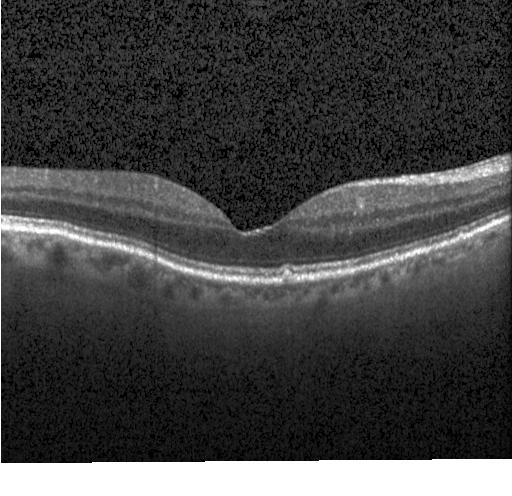
Fovea-centered, OCT line scan, spectral-domain optical coherence tomography. The scan shows neither CNV, DME, nor drusen.